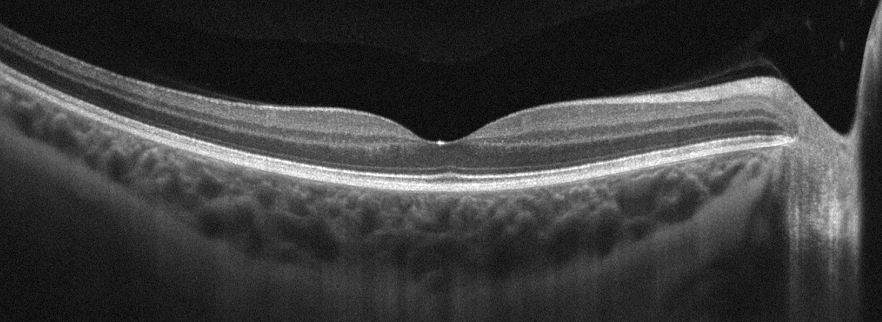

Right eye · OCT B-scan · instrument: Optovue Avanti RTVue XR. The scan shows no evidence of AMD, DME, ERM, RAO, RVO, or VID.